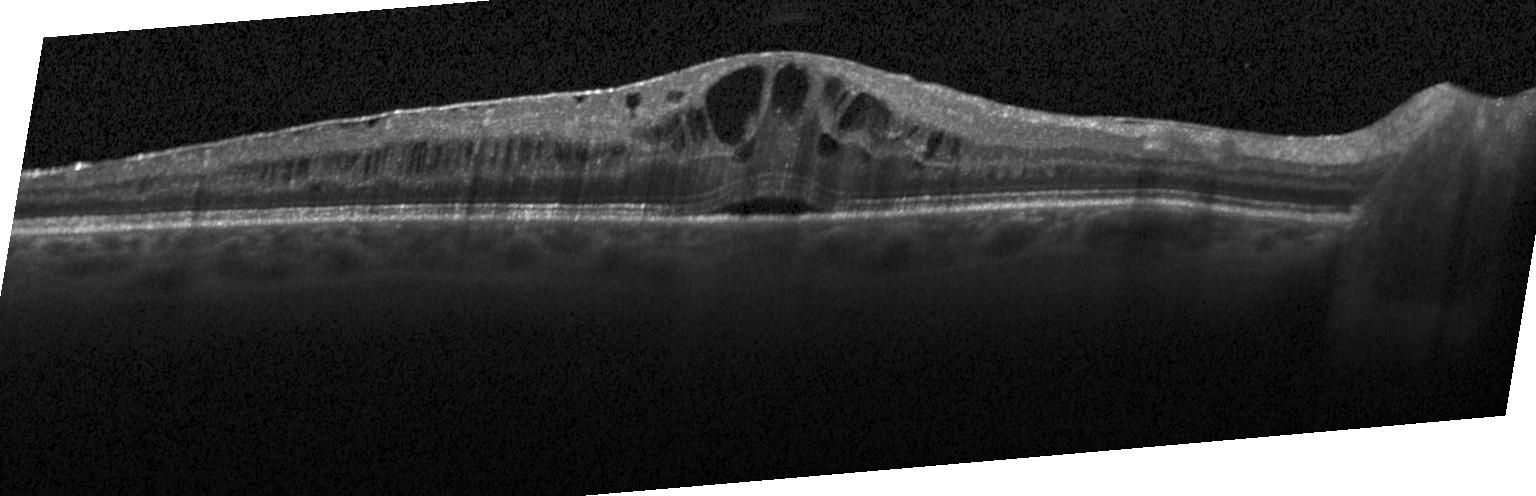

Macular OCT: diabetic macular edema.